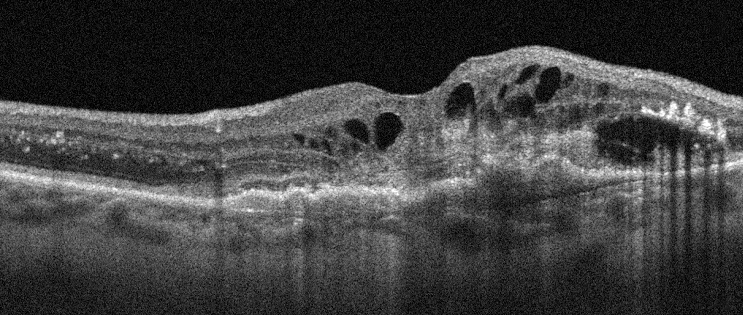 OD; OCT B-scan; fovea-centered. OCT finding: AMD.